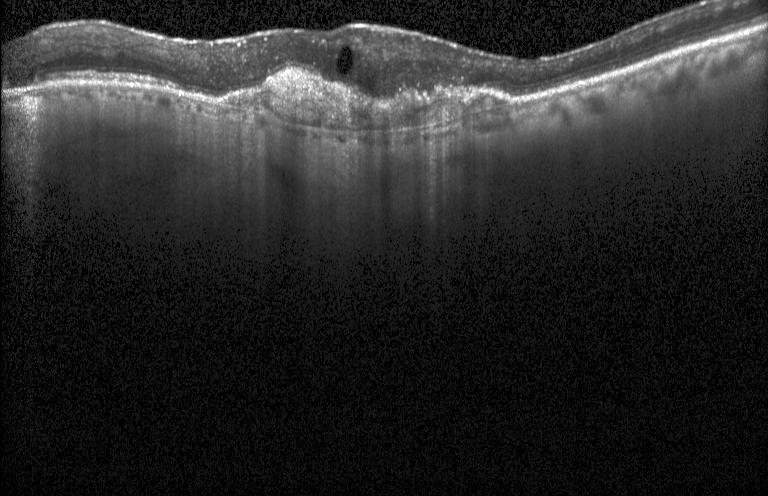

Spectral-domain OCT · optical coherence tomography scan · macular scan · instrument: Heidelberg Spectralis.
Macular OCT: CNV.